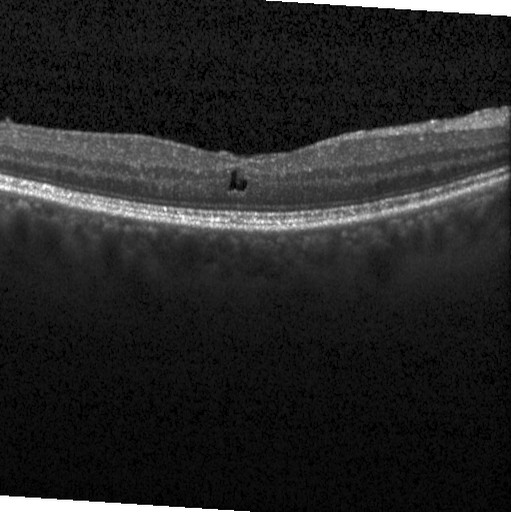

Dx: DME.